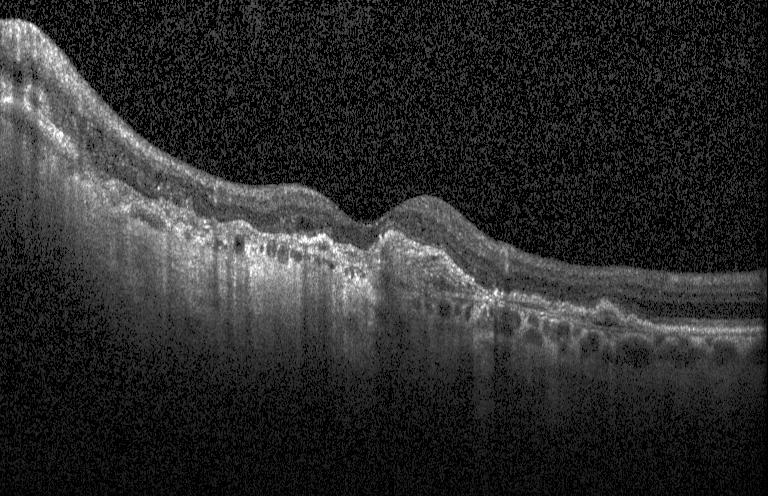 Impression: a choroidal neovascular membrane.